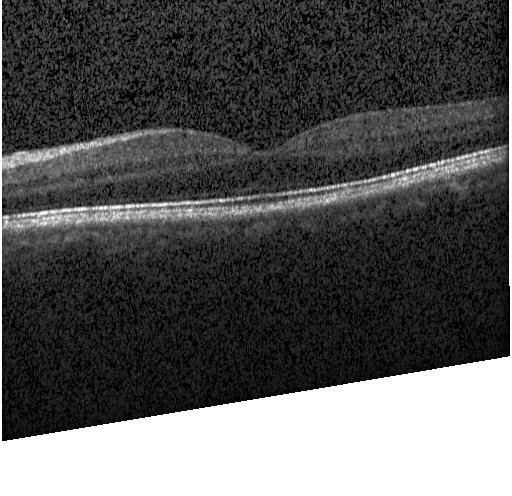
OCT B-scan — Finding: neither choroidal neovascularization, diabetic macular edema, nor drusen.